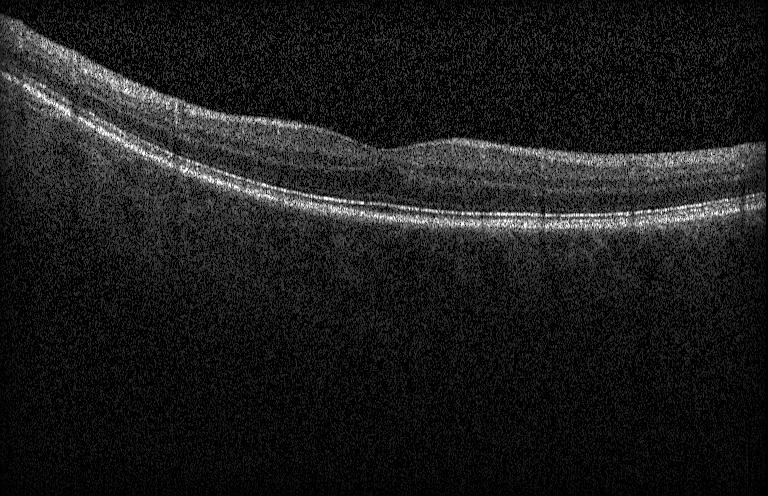
Optical coherence tomography B-scan. The scan shows no choroidal neovascularization, no diabetic macular edema, and no drusen.